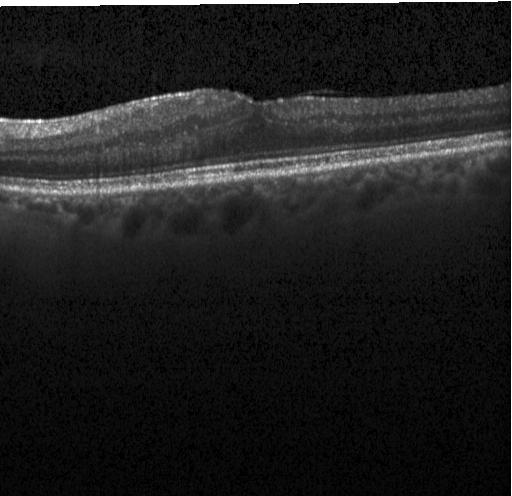

Instrument: Heidelberg Spectralis, SD-OCT, macular scan, retinal OCT cross-section — Macular OCT: no choroidal neovascularization, diabetic macular edema, or drusen.